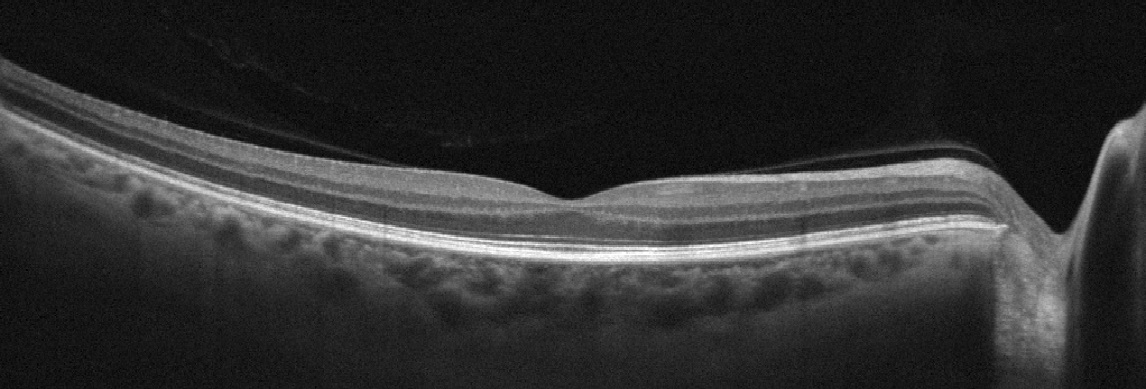 Retinal OCT cross-section. Impression: no evidence of AMD, DME, ERM, RAO, RVO, or VID.